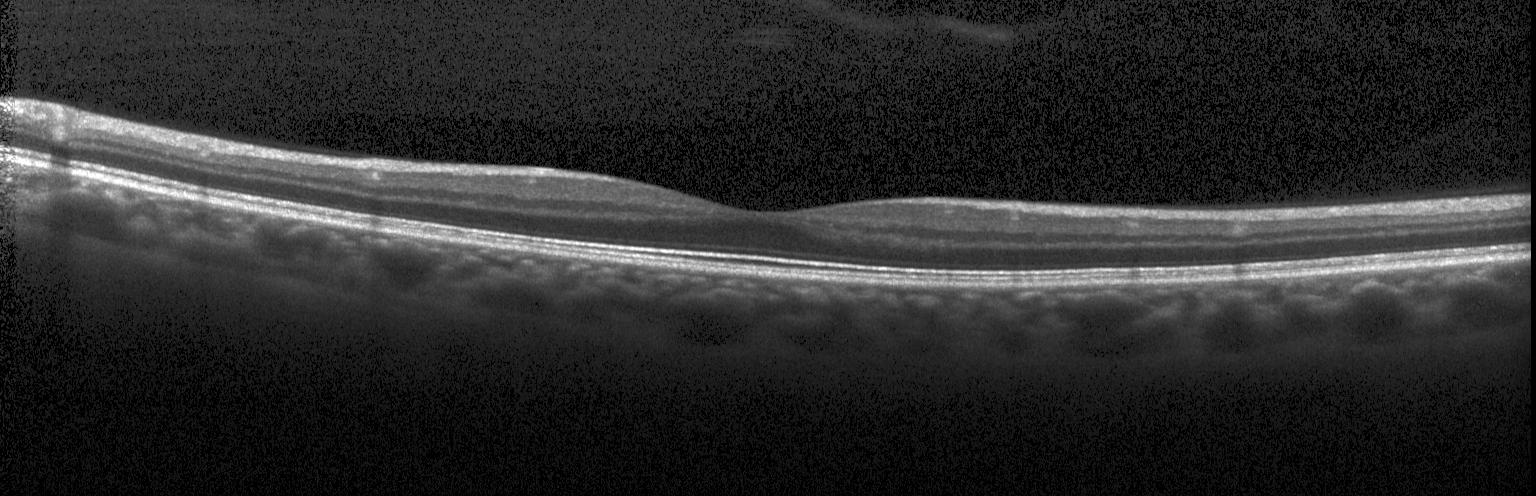 Diagnosis: no evidence of choroidal neovascularization, diabetic macular edema, or drusen.